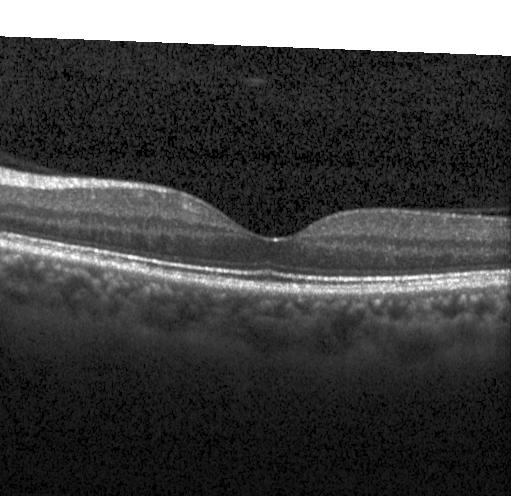

Heidelberg Spectralis OCT system, optical coherence tomography scan, horizontal scan through the fovea, spectral-domain OCT.
This B-scan demonstrates neither choroidal neovascularization, diabetic macular edema, nor drusen.